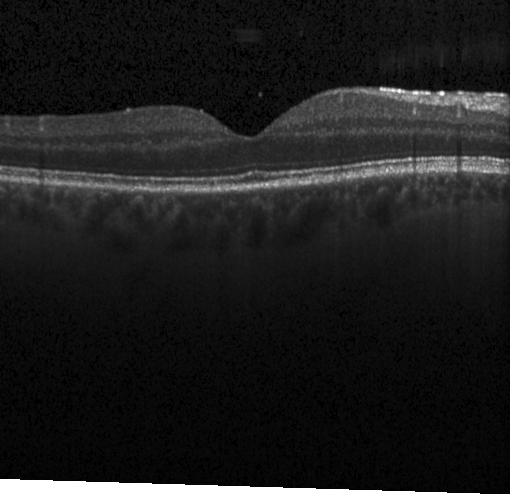
Spectral-domain OCT · retinal OCT cross-section — Assessment: no choroidal neovascularization, no diabetic macular edema, and no drusen.